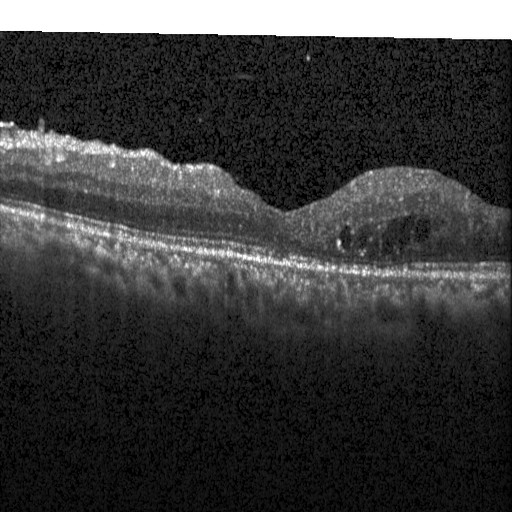 OCT line scan · SD-OCT · acquired on a Heidelberg Spectralis · fovea-centered.
This B-scan demonstrates diabetic macular edema (DME).